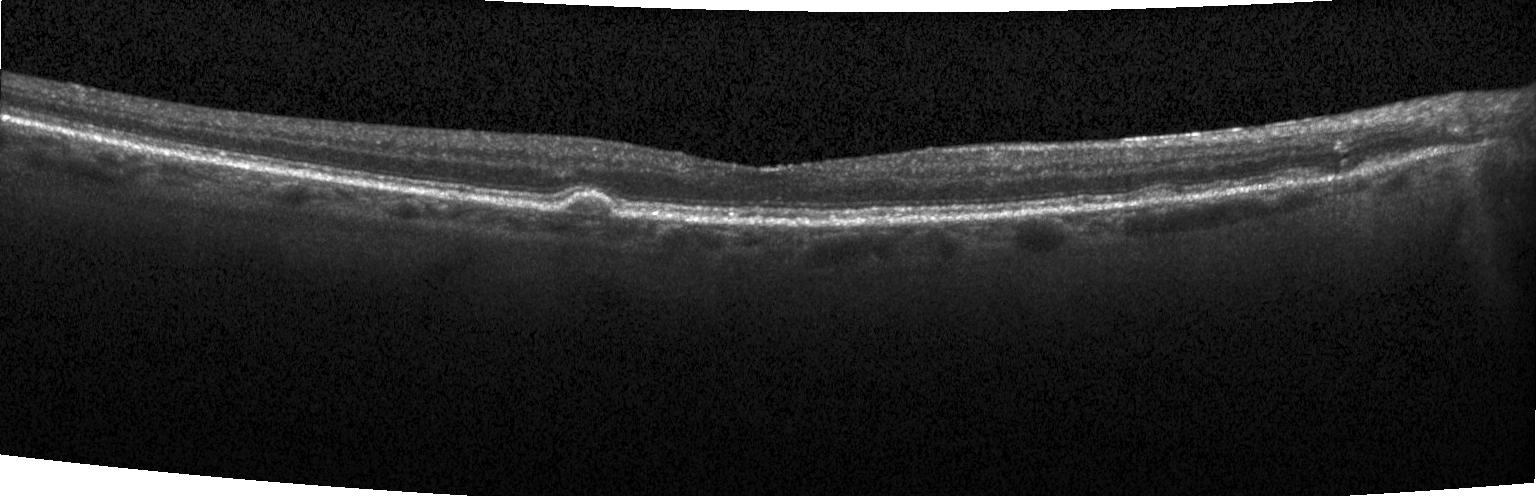
Retinal OCT B-scan. Macular scan. Heidelberg Spectralis OCT system — Impression: sub-RPE drusenoid deposits.